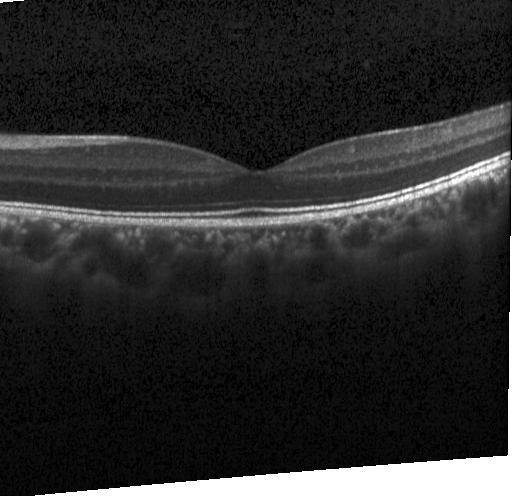
Macular OCT demonstrating neither choroidal neovascularization, diabetic macular edema, nor drusen.